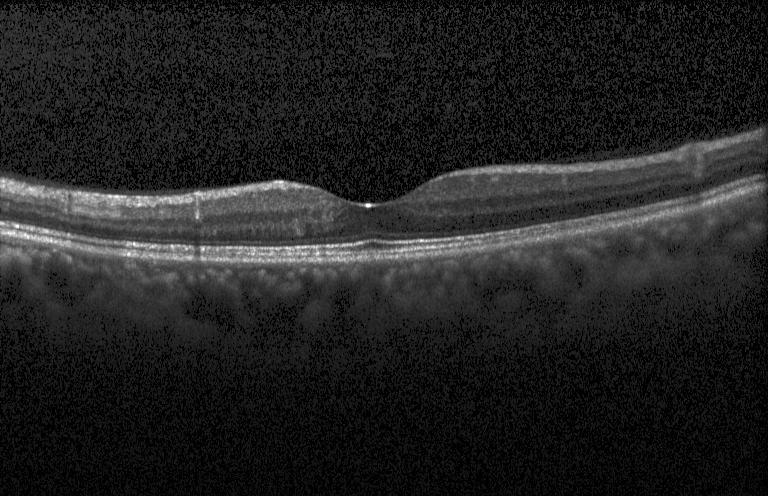 OCT line scan — This B-scan demonstrates neither CNV, DME, nor drusen.